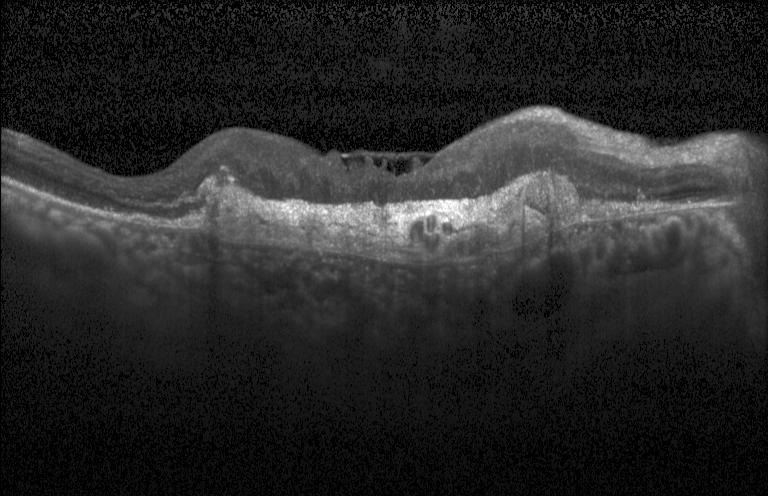 Finding: a choroidal neovascular membrane.